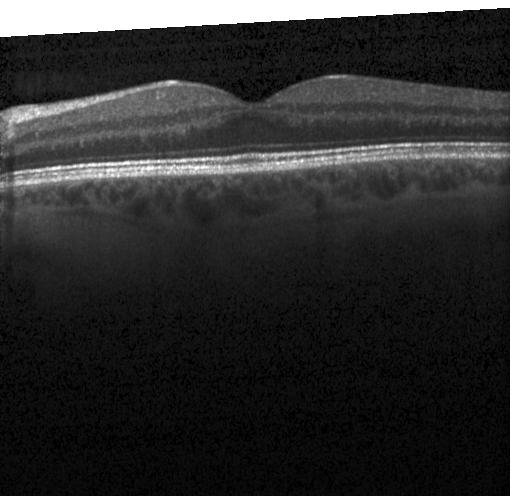 Retinal OCT B-scan. Through the macula
No choroidal neovascularization, diabetic macular edema, or drusen.